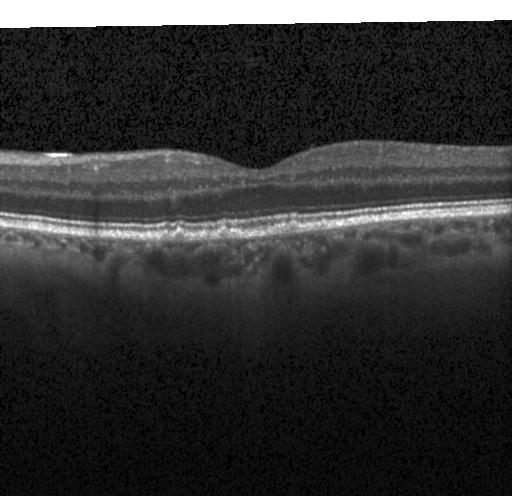
Heidelberg Spectralis OCT system, horizontal scan through the fovea, OCT B-scan
Sub-RPE drusenoid deposits.